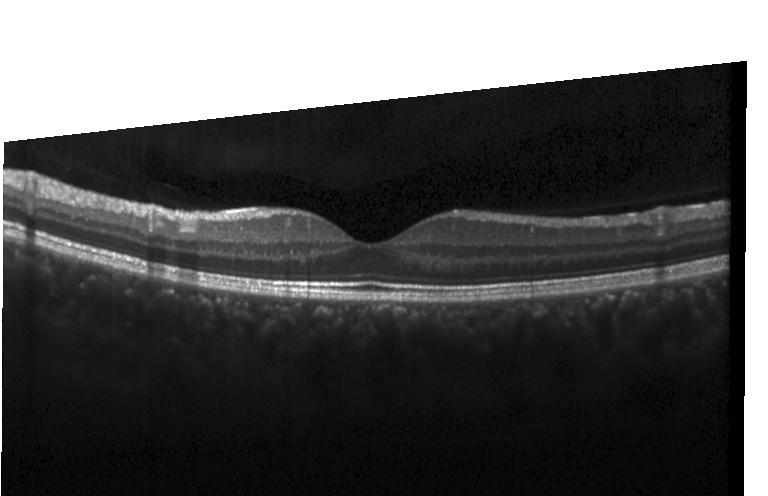
Dx: no choroidal neovascularization, no diabetic macular edema, and no drusen.